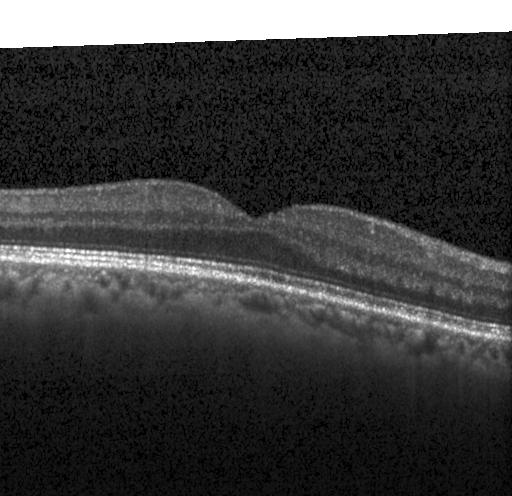

SD-OCT; optical coherence tomography scan; centered on the fovea. Diagnosis: no CNV, no DME, and no drusen.